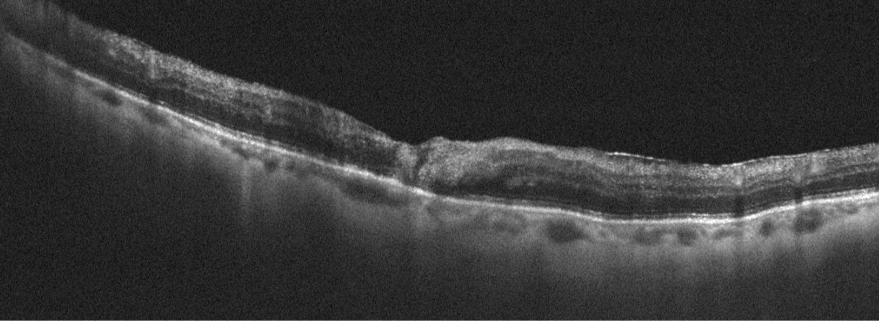
Optical coherence tomography scan. Macular scan. Acquired on an Optovue Avanti RTVue XR.
Finding: diabetic macular edema (DME).